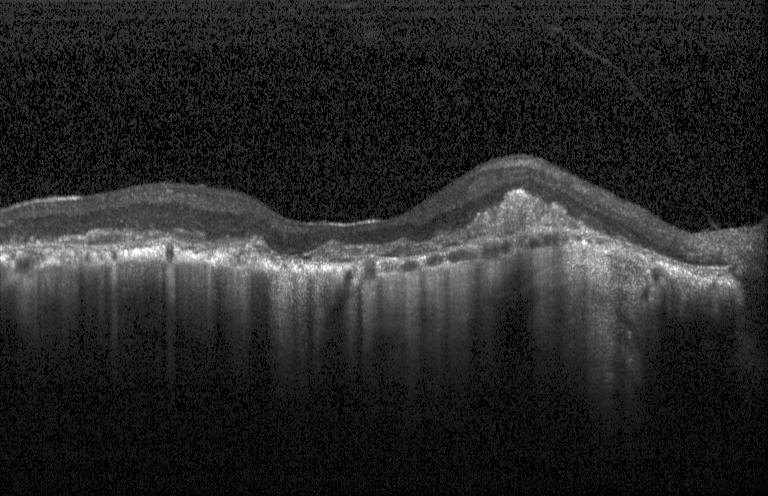
A choroidal neovascular membrane.